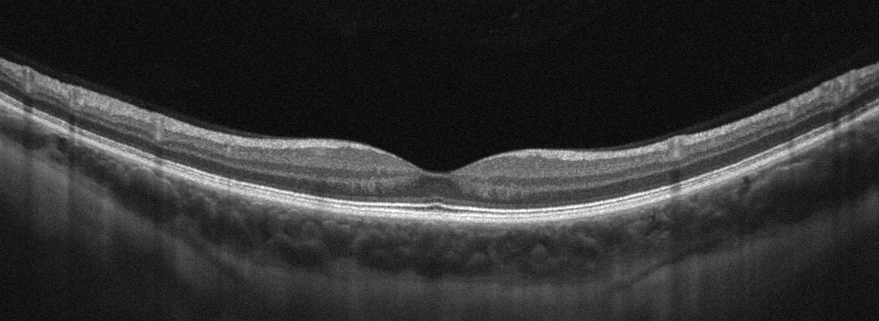
Retinal OCT B-scan — Diagnosis: no AMD, DME, ERM, RAO, RVO, or VID.